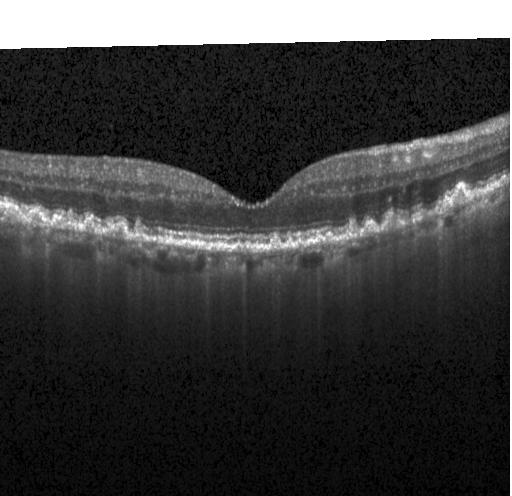
Through the macula, OCT B-scan.
The scan shows sub-RPE drusenoid deposits.